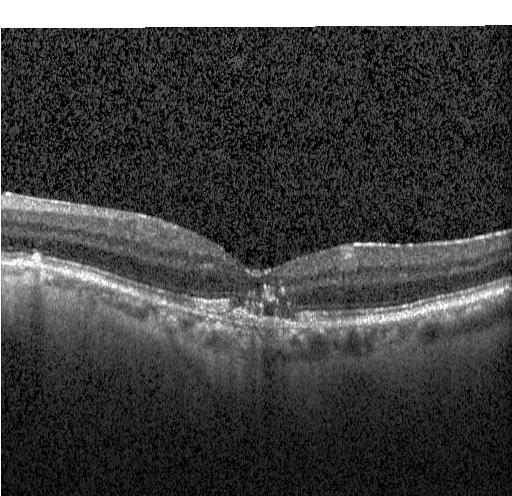

Retinal OCT B-scan; horizontal scan through the fovea — OCT finding: choroidal neovascularization.